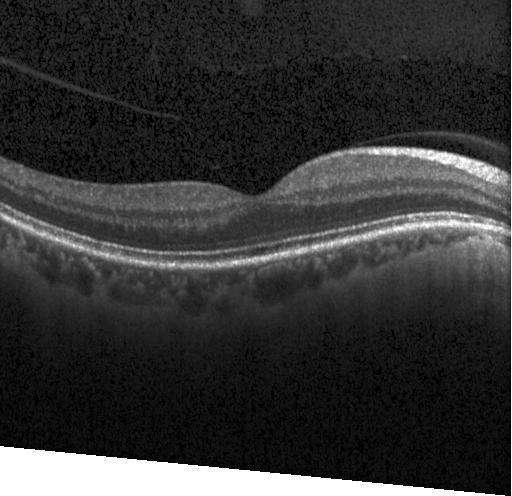

Heidelberg Spectralis, OCT line scan, centered on the fovea, spectral-domain OCT — OCT finding: no CNV, DME, or drusen.